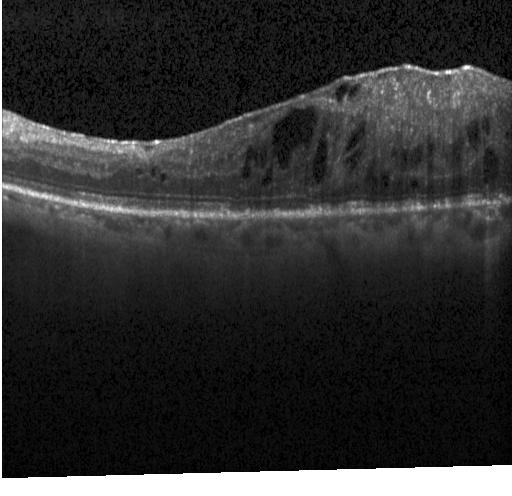

Diabetic macular edema (DME).